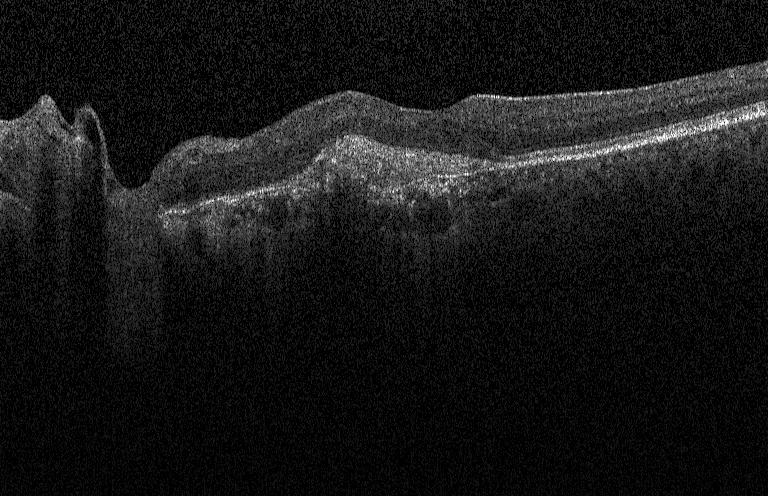 OCT B-scan — The scan shows a choroidal neovascular membrane.